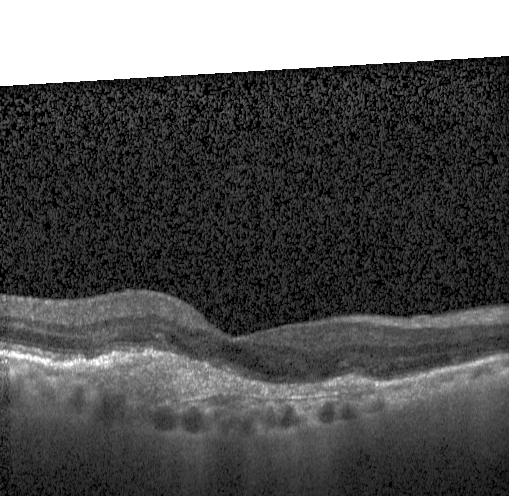
OCT B-scan. Impression: a choroidal neovascular membrane.